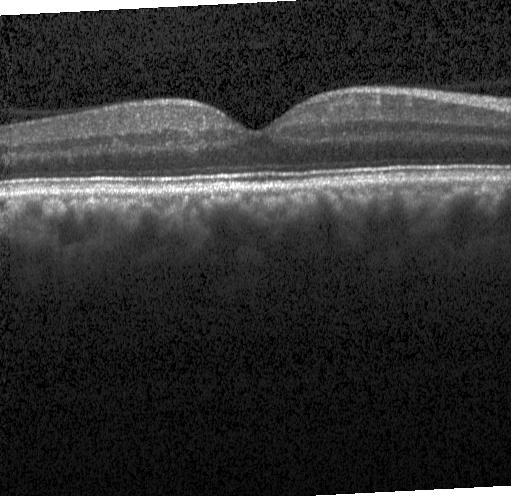

Diagnosis: neither CNV, DME, nor drusen.